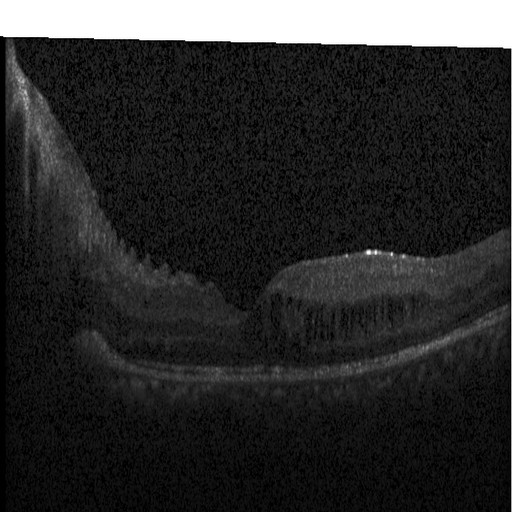 OCT B-scan.
Macular OCT: diabetic macular edema.